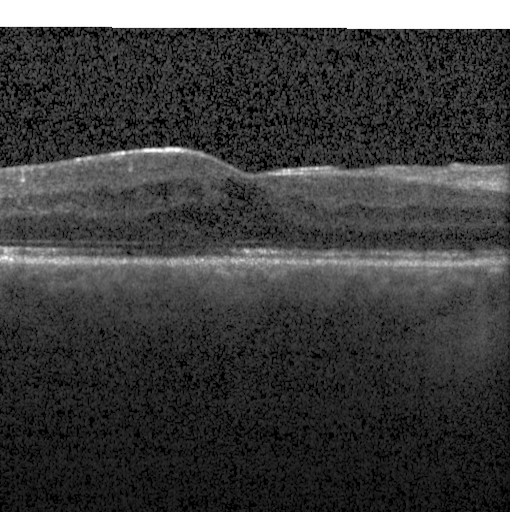

Optical coherence tomography B-scan
Impression: DME.